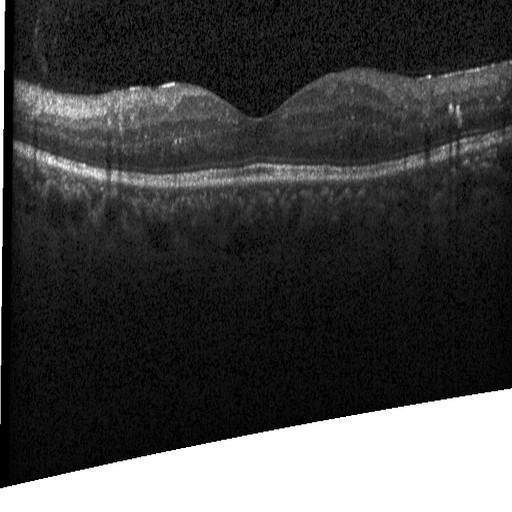

Assessment: diabetic macular edema (DME).